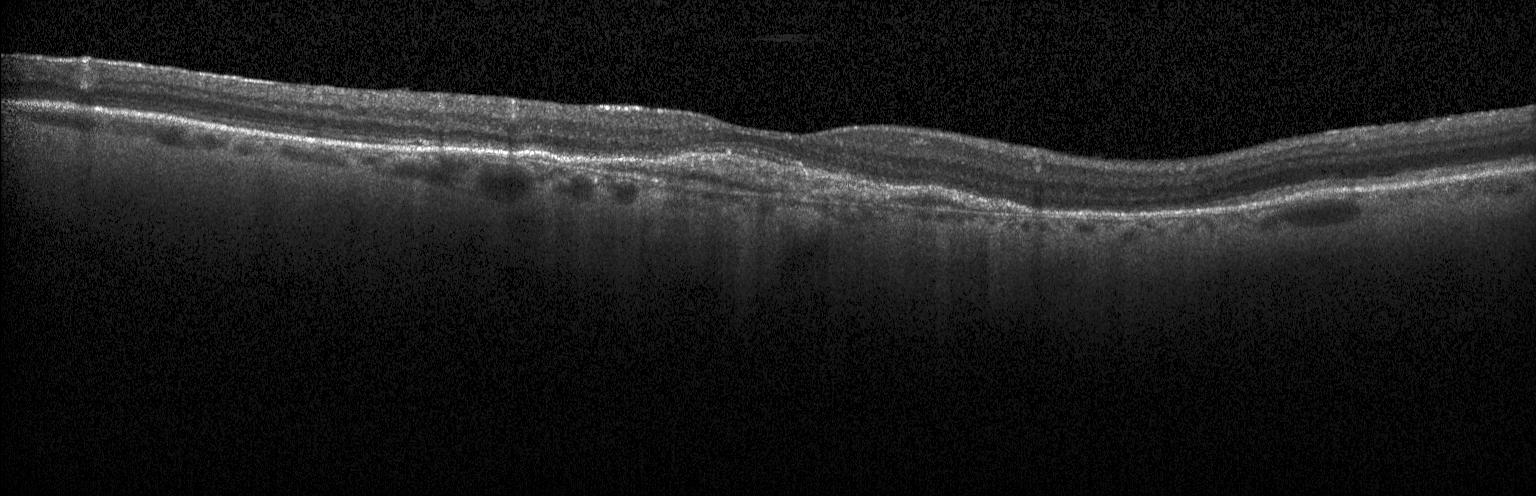 Diagnosis: a choroidal neovascular membrane.